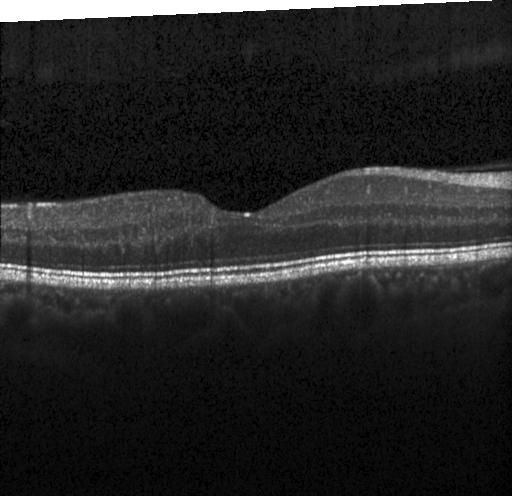 SD-OCT · Heidelberg Spectralis OCT system · OCT B-scan. Diagnosis: no evidence of choroidal neovascularization, diabetic macular edema, or drusen.